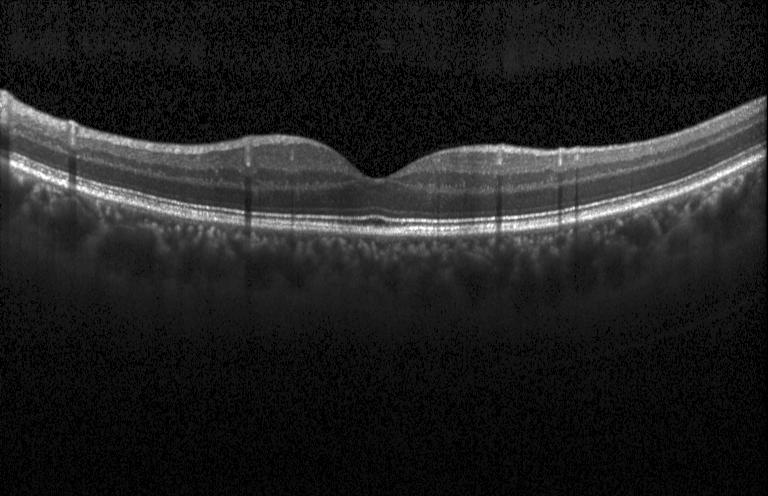 No evidence of choroidal neovascularization, diabetic macular edema, or drusen.